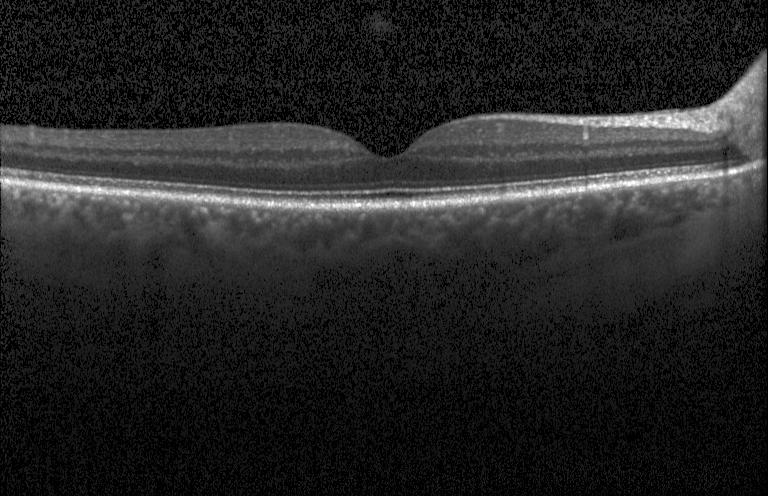 Spectral-domain OCT; OCT B-scan — Finding: no evidence of choroidal neovascularization, diabetic macular edema, or drusen.